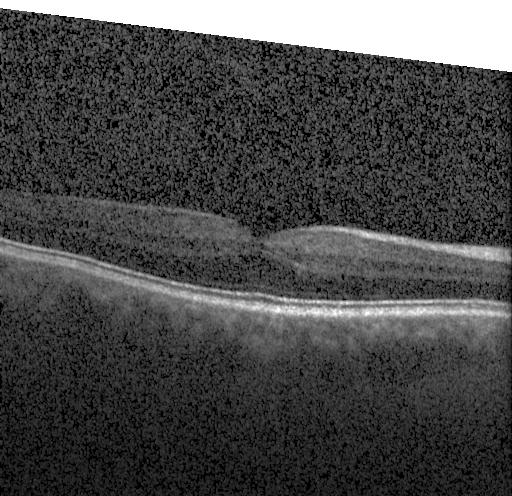

Spectral-domain optical coherence tomography. Heidelberg Spectralis. OCT line scan. Fovea-centered.
Macular OCT: no choroidal neovascularization, diabetic macular edema, or drusen.